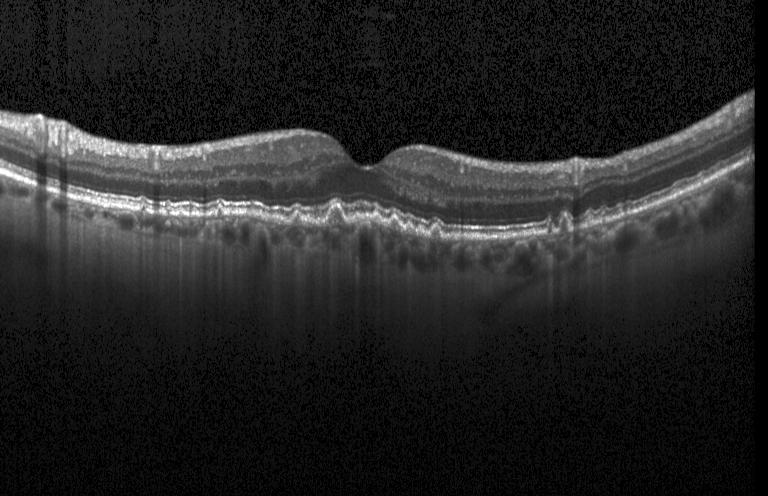 Optical coherence tomography scan, spectral-domain optical coherence tomography
Diagnosis: multiple drusen.